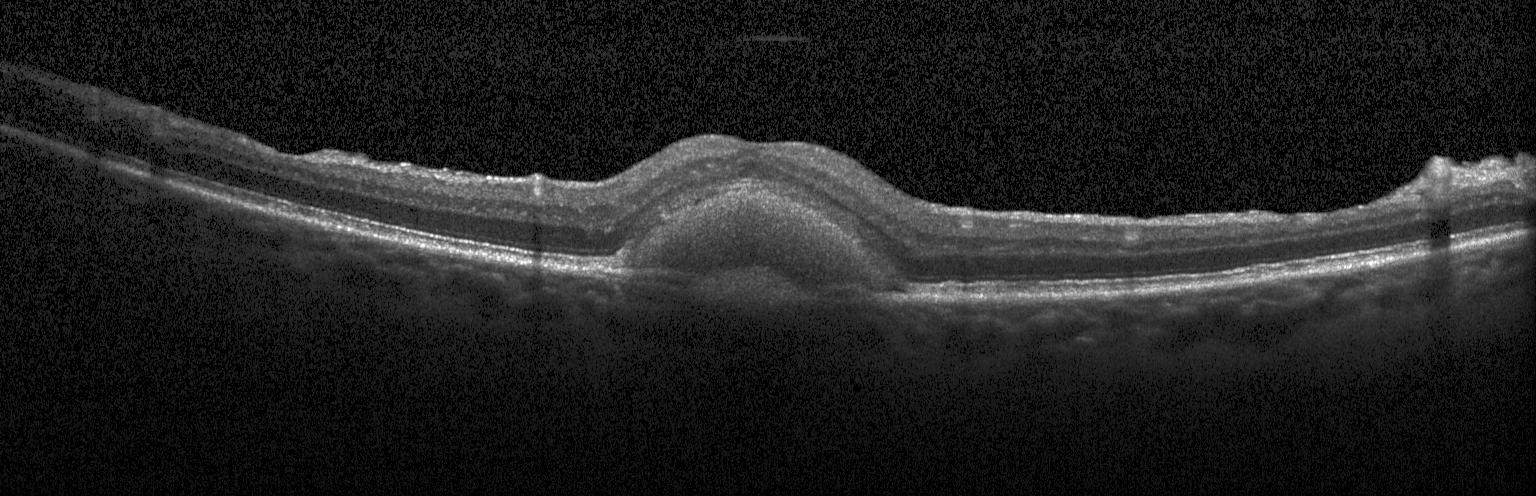
Optical coherence tomography B-scan
Macular OCT: a choroidal neovascular membrane.